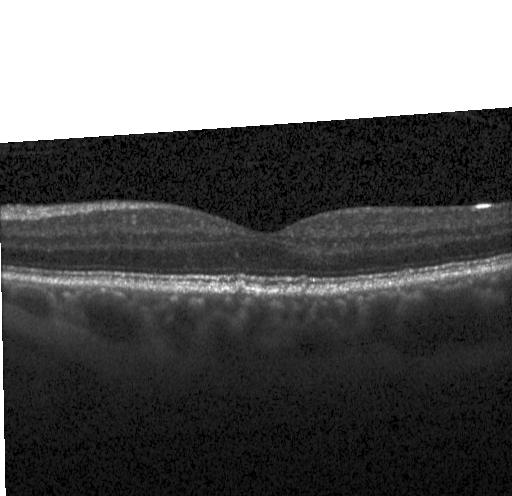

Retinal OCT cross-section — Diagnosis: sub-RPE drusenoid deposits.